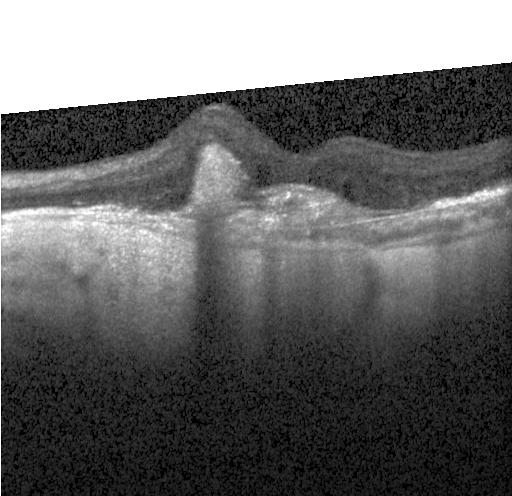 OCT line scan · acquired on a Heidelberg Spectralis · SD-OCT — OCT finding: a choroidal neovascular membrane.